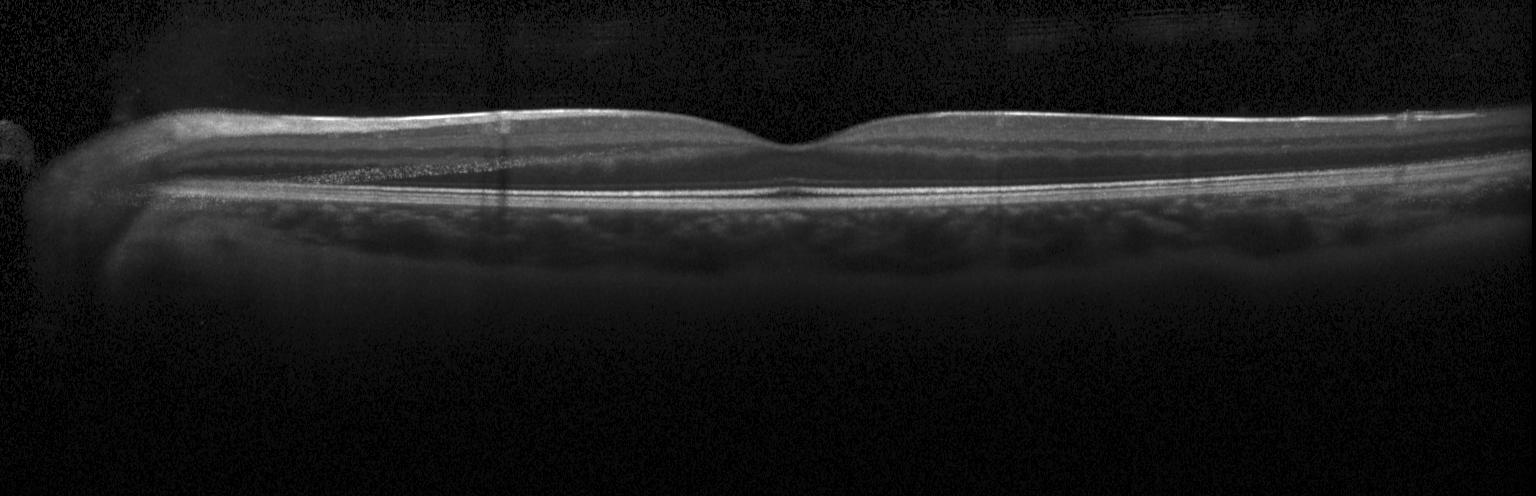 Finding: no evidence of choroidal neovascularization, diabetic macular edema, or drusen.